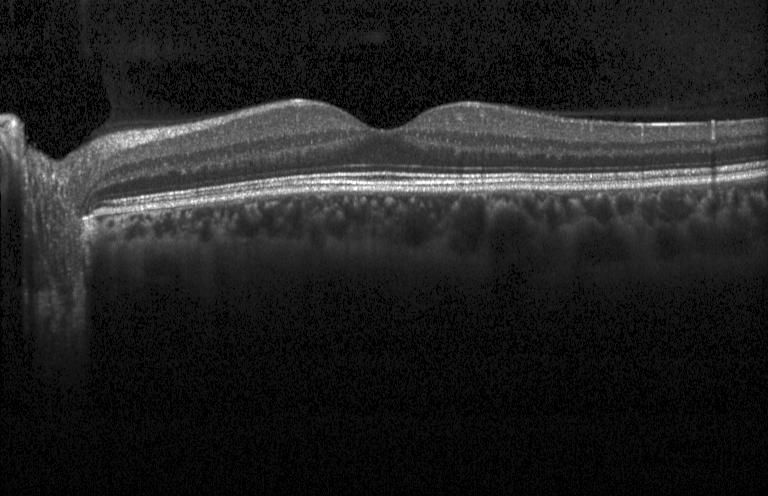

Finding: neither CNV, DME, nor drusen.